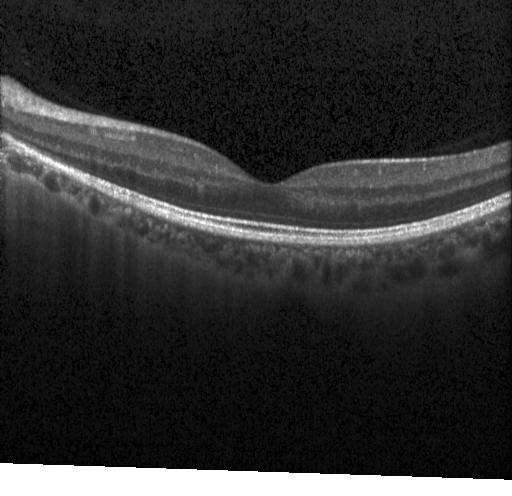 Finding: no choroidal neovascularization, diabetic macular edema, or drusen.